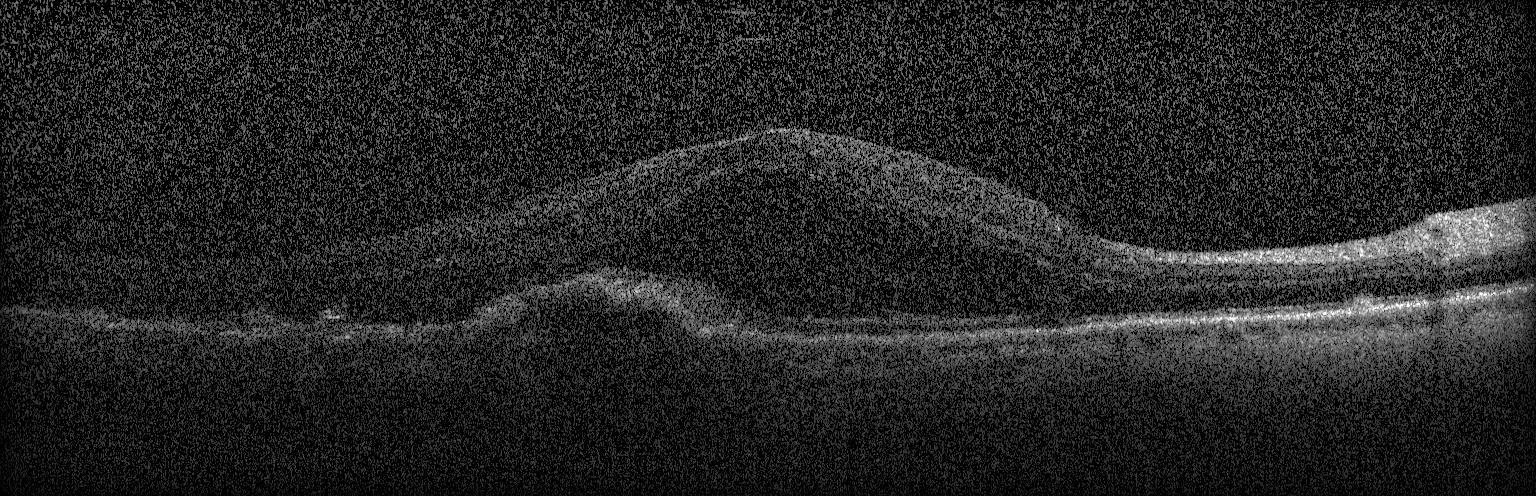

Dx: a choroidal neovascular membrane.